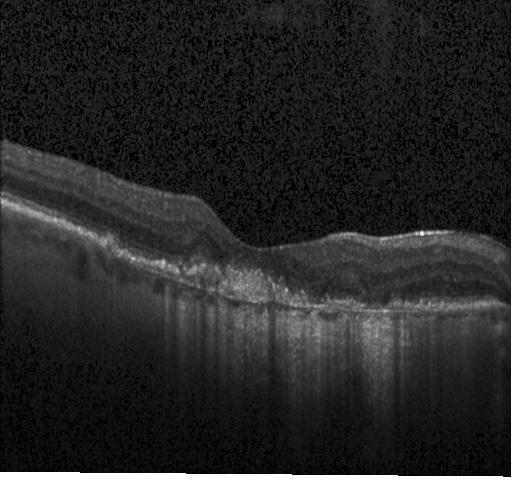
Finding: choroidal neovascularization.